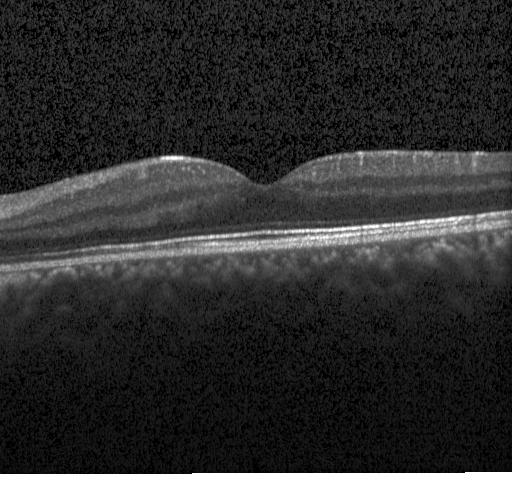
Dx: no choroidal neovascularization, no diabetic macular edema, and no drusen.